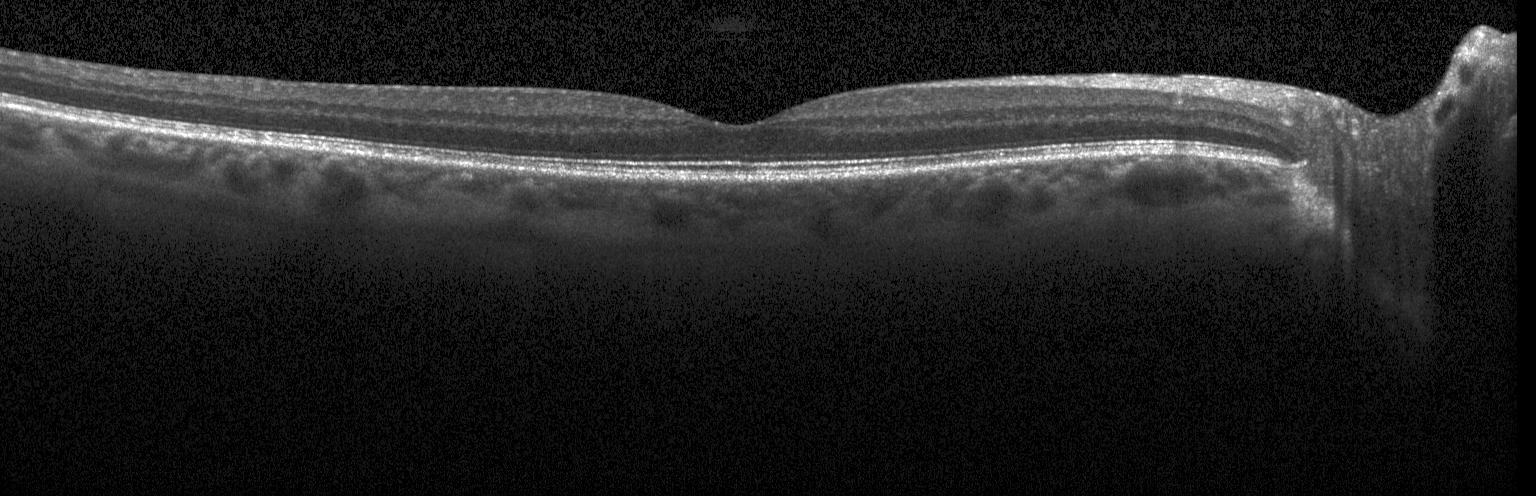

Diagnosis: no choroidal neovascularization, diabetic macular edema, or drusen.